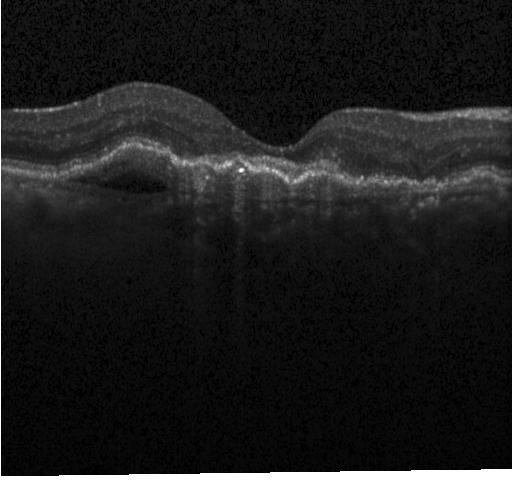 Through the macula. OCT line scan.
This B-scan demonstrates choroidal neovascularization.